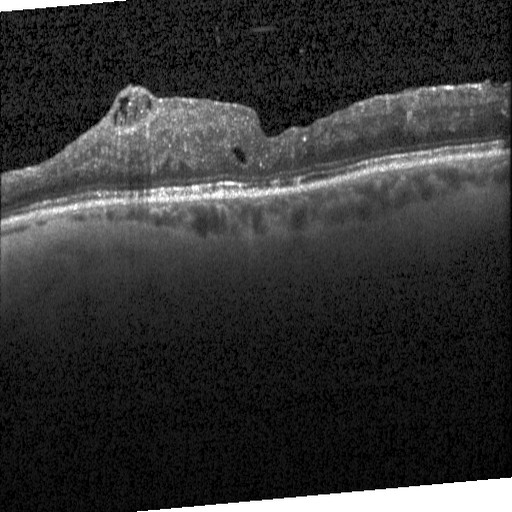

Centered on the fovea · OCT B-scan · spectral-domain OCT · Heidelberg Spectralis OCT system — The scan shows diabetic macular edema (DME).